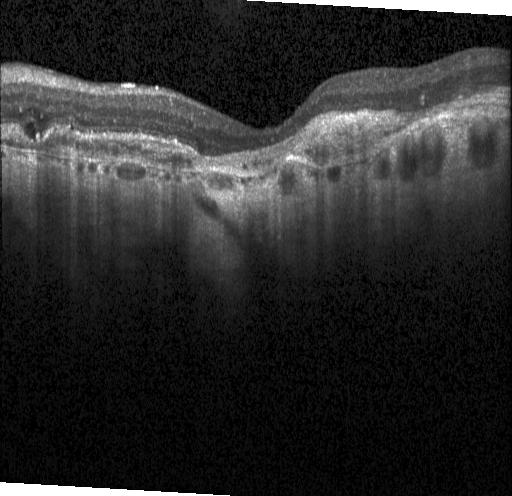

OCT line scan
Impression: choroidal neovascularization (CNV).